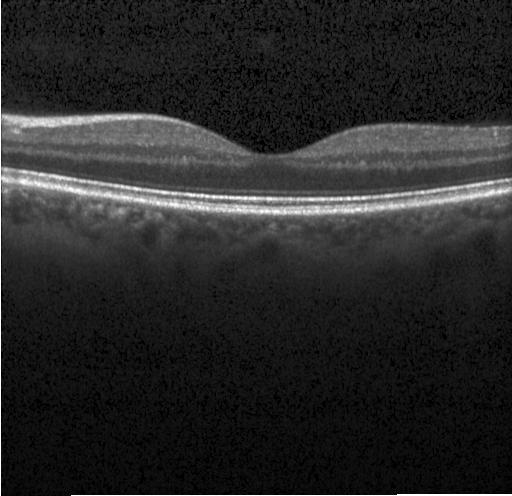
Macular scan, optical coherence tomography B-scan, acquired on a Heidelberg Spectralis, spectral-domain OCT.
Impression: no evidence of choroidal neovascularization, diabetic macular edema, or drusen.